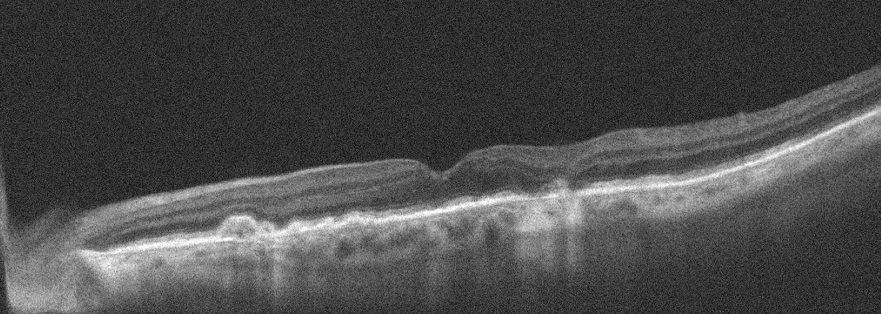
Optical coherence tomography scan
Assessment: age-related macular degeneration.